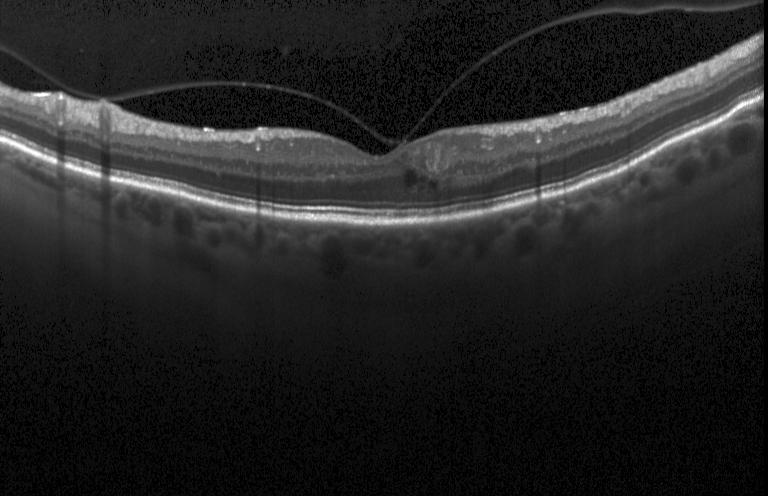 Fovea-centered. Heidelberg Spectralis OCT system. Optical coherence tomography scan. SD-OCT — Finding: diabetic macular edema.